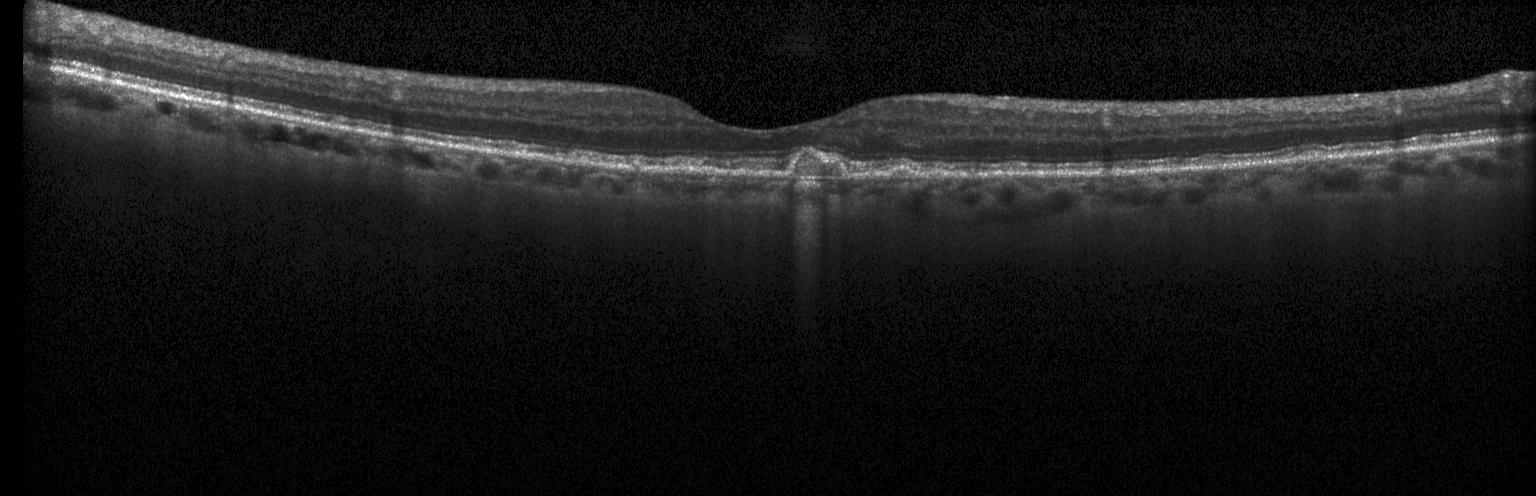
Finding: sub-RPE drusenoid deposits.